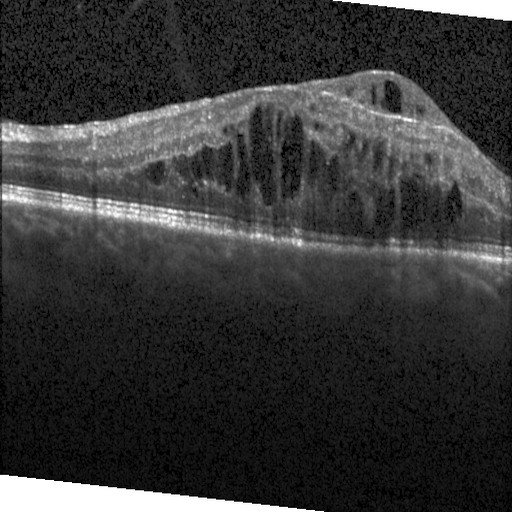 Diagnosis: diabetic macular edema.